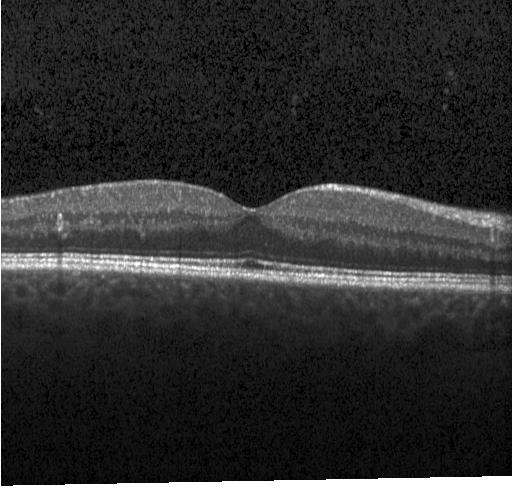

Spectral-domain OCT · OCT B-scan
Diagnosis: no choroidal neovascularization, diabetic macular edema, or drusen.